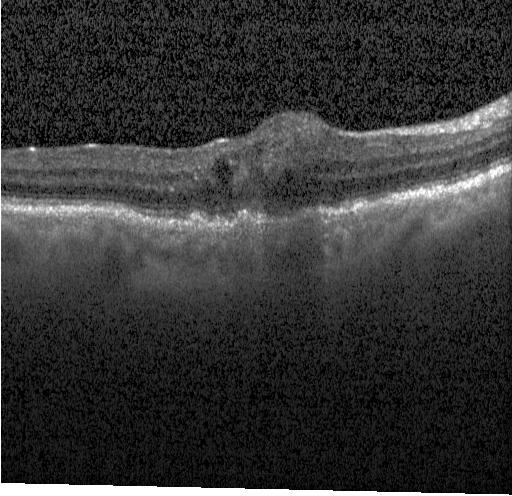

SD-OCT, acquired on a Heidelberg Spectralis, retinal OCT B-scan
Assessment: CNV.